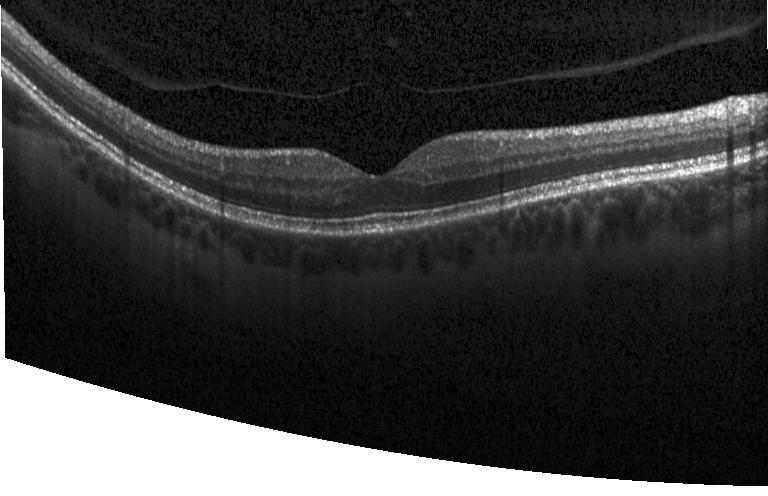

Retinal OCT cross-section. Fovea-centered. Heidelberg Spectralis. Spectral-domain optical coherence tomography
Diagnosis: no choroidal neovascularization, no diabetic macular edema, and no drusen.